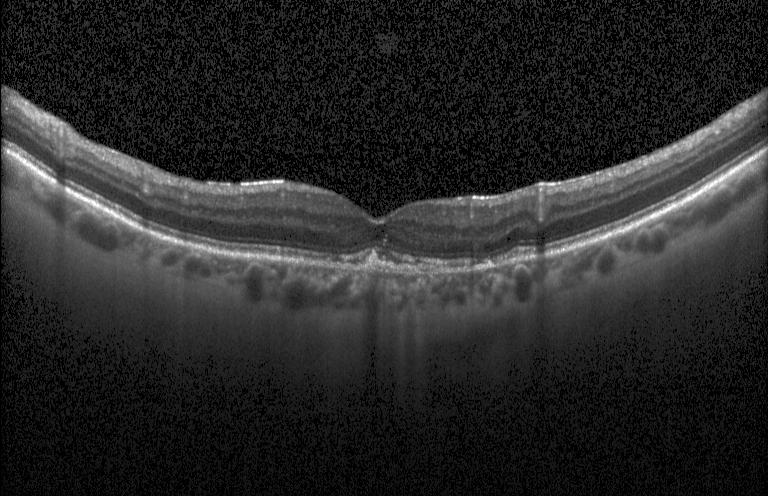
Spectral-domain OCT B-scan: choroidal neovascularization.